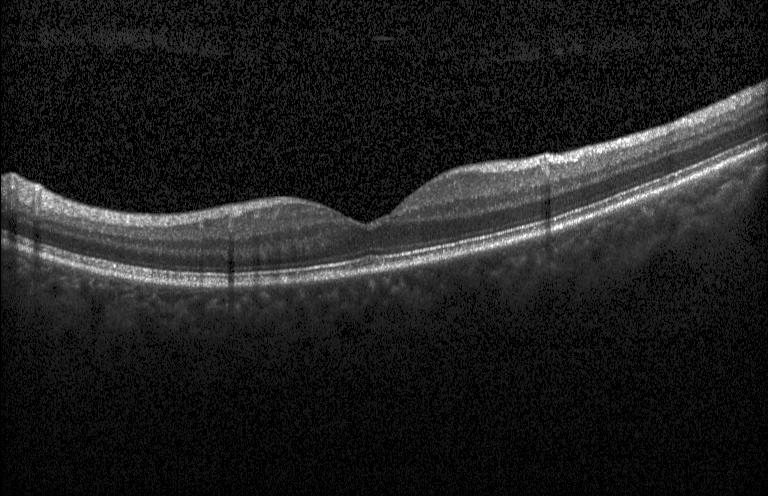

Optical coherence tomography scan — Impression: no evidence of choroidal neovascularization, diabetic macular edema, or drusen.